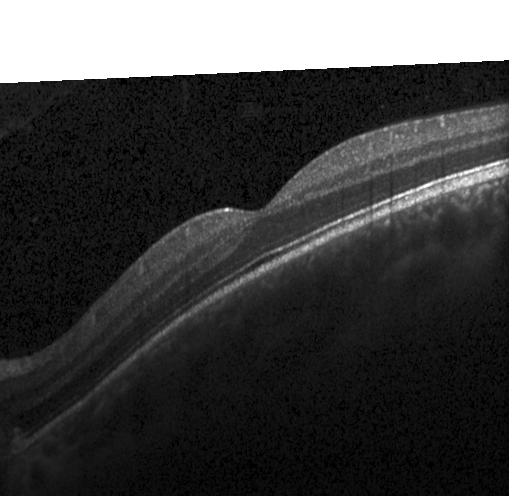

Macular OCT demonstrating no choroidal neovascularization, diabetic macular edema, or drusen.